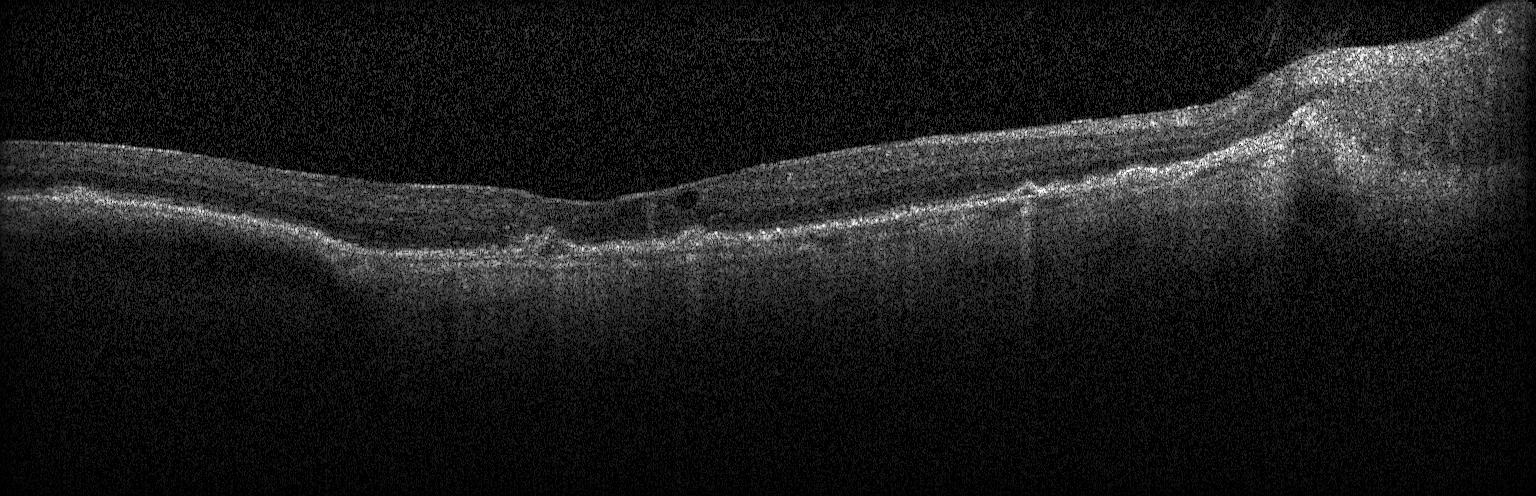

Acquired on a Heidelberg Spectralis, spectral-domain OCT, OCT B-scan. OCT finding: a choroidal neovascular membrane.